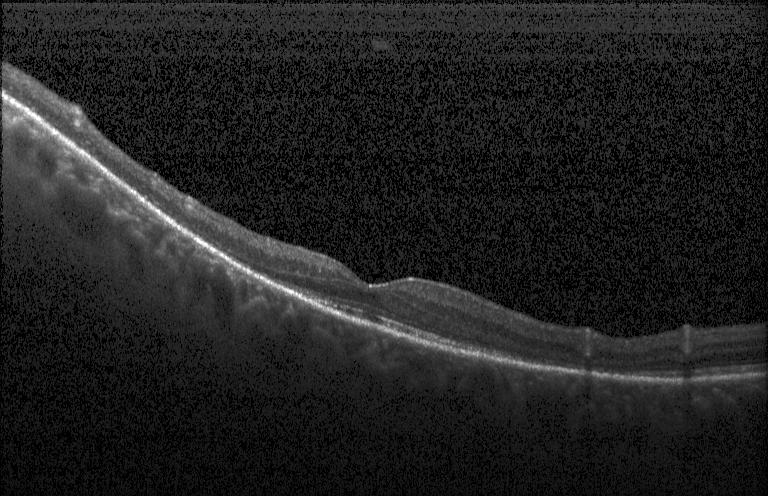
Impression: no CNV, DME, or drusen.